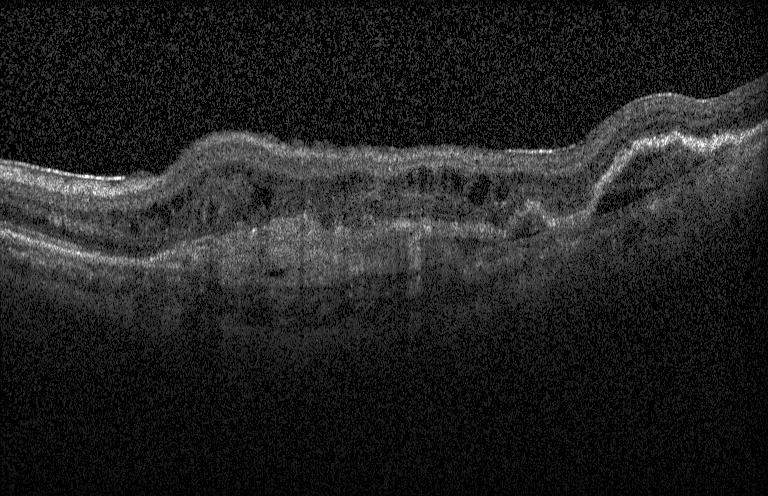

Impression: choroidal neovascularization.